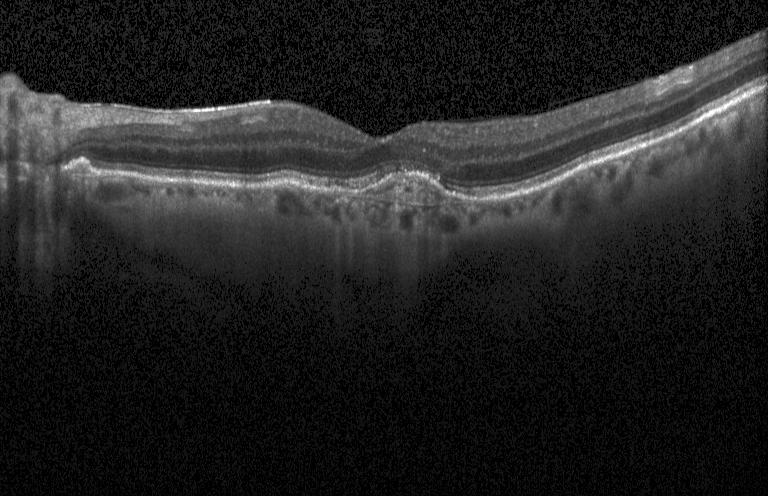 Impression: CNV.